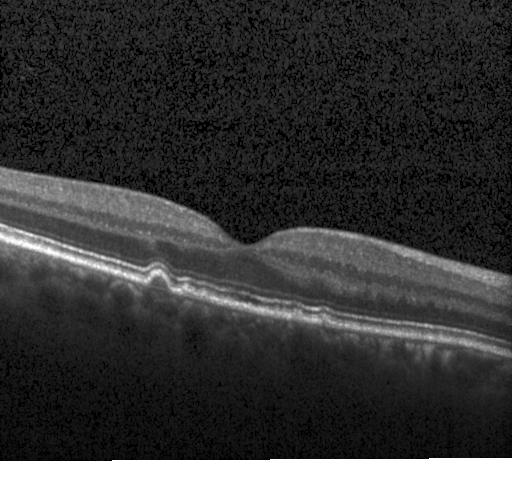

Assessment: sub-RPE drusenoid deposits.